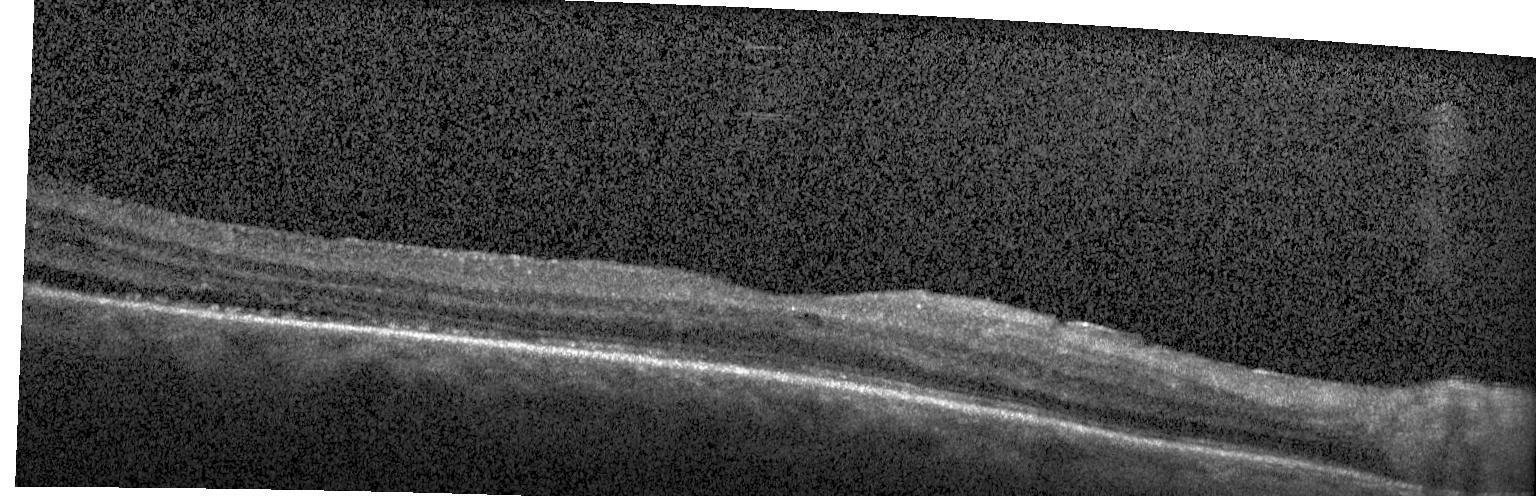 Through the macula · OCT line scan
Impression: diabetic macular edema (DME).